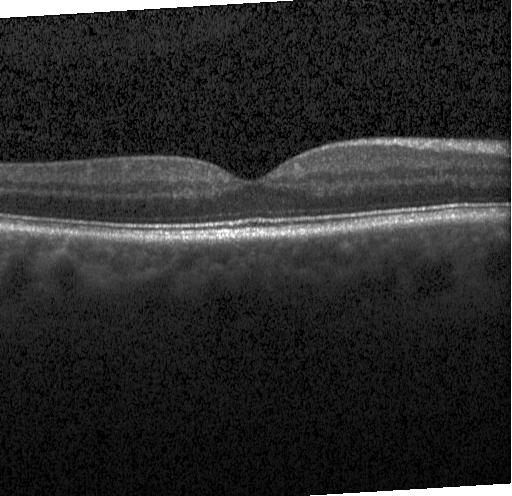
Optical coherence tomography B-scan — The scan shows no evidence of choroidal neovascularization, diabetic macular edema, or drusen.